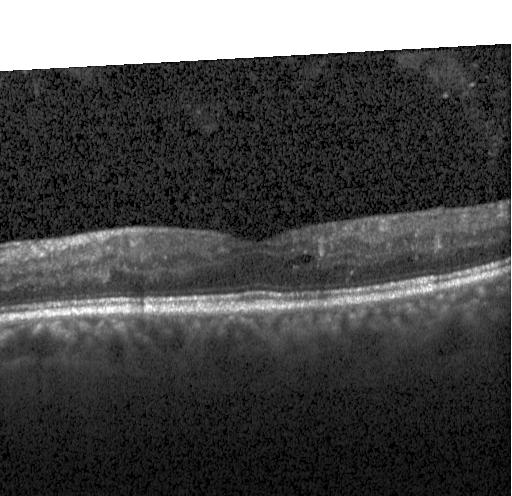

Heidelberg Spectralis OCT system. Spectral-domain OCT. OCT line scan. Diagnosis: diabetic macular edema (DME).